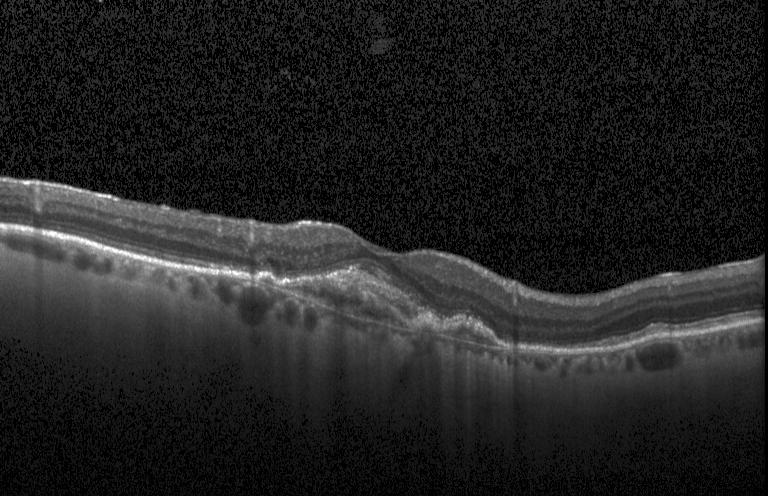

Spectral-domain OCT; fovea-centered; retinal OCT cross-section; instrument: Heidelberg Spectralis
Finding: choroidal neovascularization (CNV).